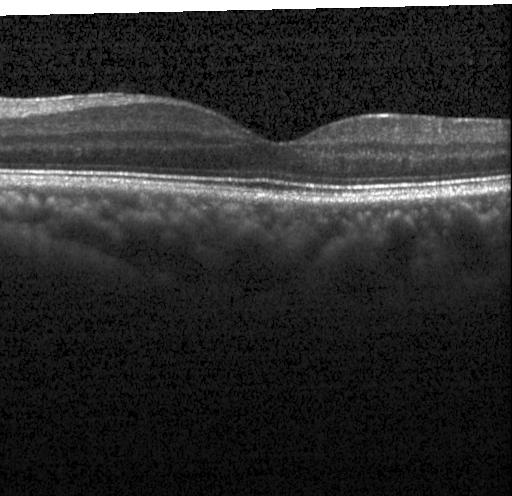
Retinal OCT cross-section · Heidelberg Spectralis · SD-OCT · macular scan — Macular OCT: no choroidal neovascularization, no diabetic macular edema, and no drusen.